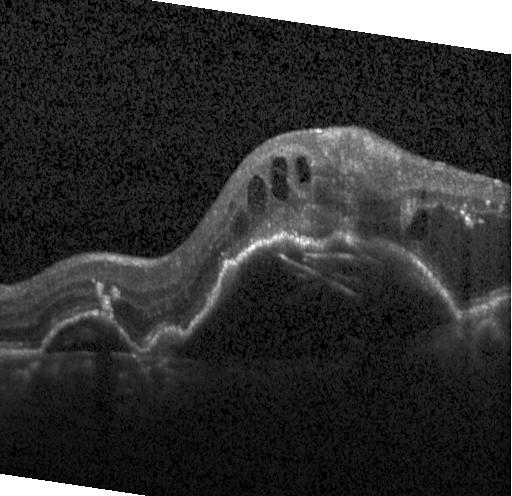 SD-OCT. Optical coherence tomography B-scan.
Dx: a choroidal neovascular membrane.